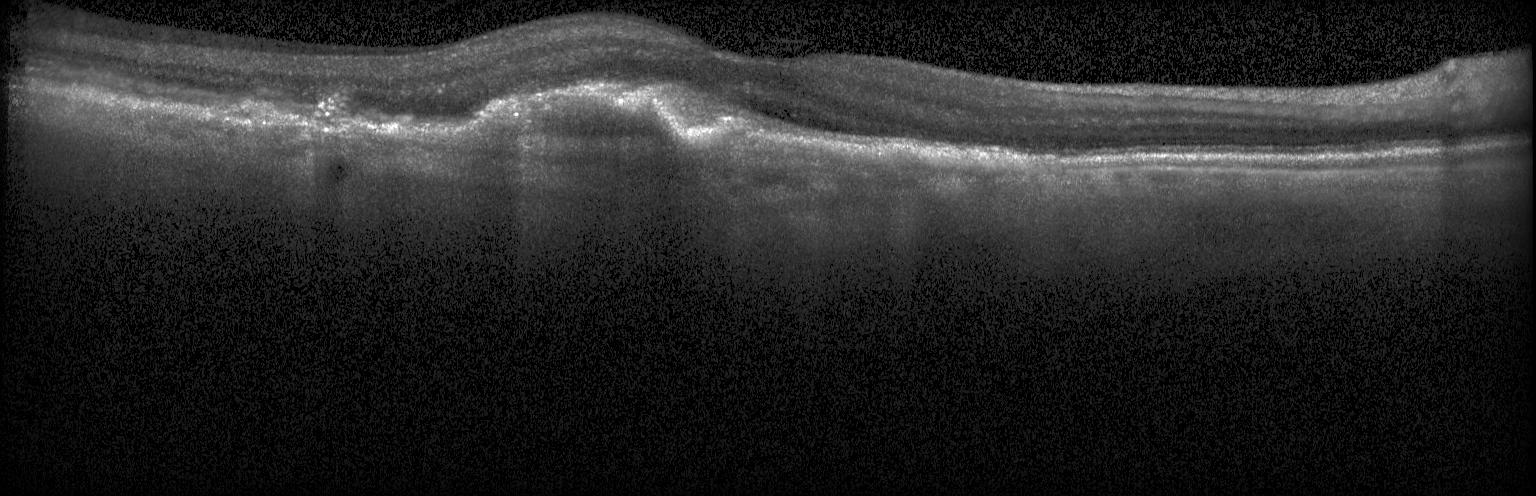
OCT finding: choroidal neovascularization (CNV).